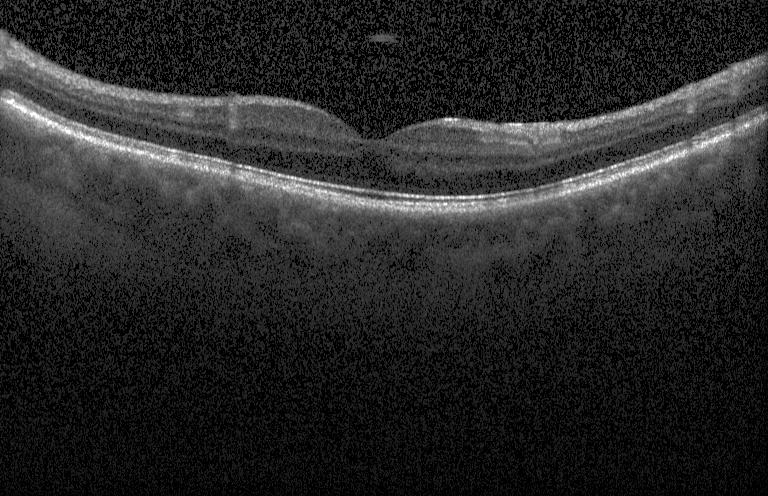 The scan shows neither choroidal neovascularization, diabetic macular edema, nor drusen.